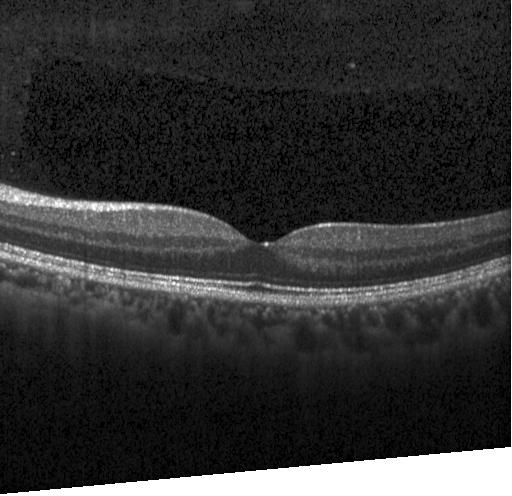
Macular scan · instrument: Heidelberg Spectralis · optical coherence tomography scan · spectral-domain OCT — Impression: no choroidal neovascularization, no diabetic macular edema, and no drusen.